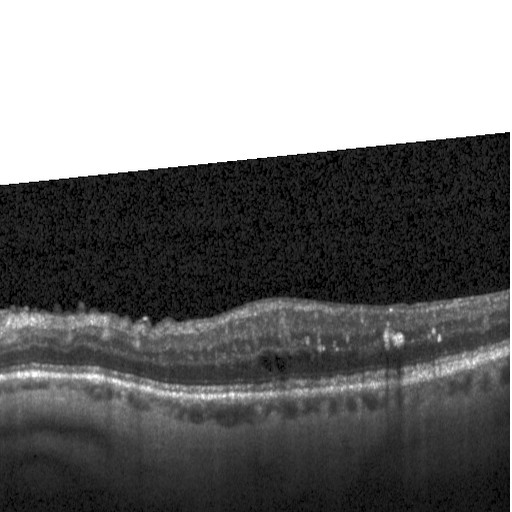

Spectral-domain optical coherence tomography. Fovea-centered. Optical coherence tomography scan — Assessment: diabetic macular edema.